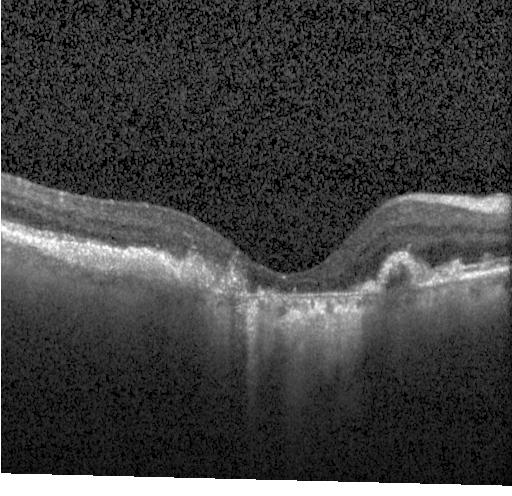
Retinal OCT cross-section showing choroidal neovascularization.